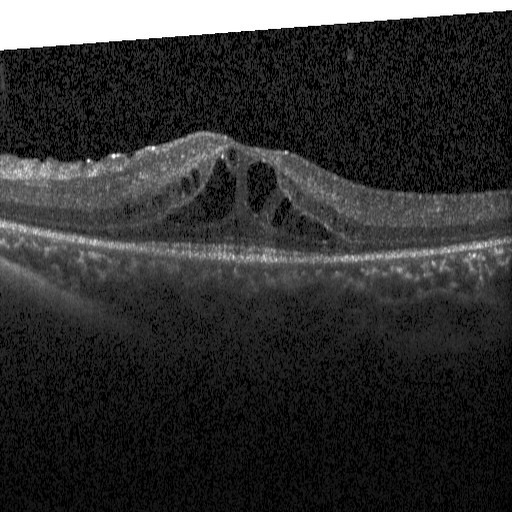

OCT B-scan showing diabetic macular edema (DME).